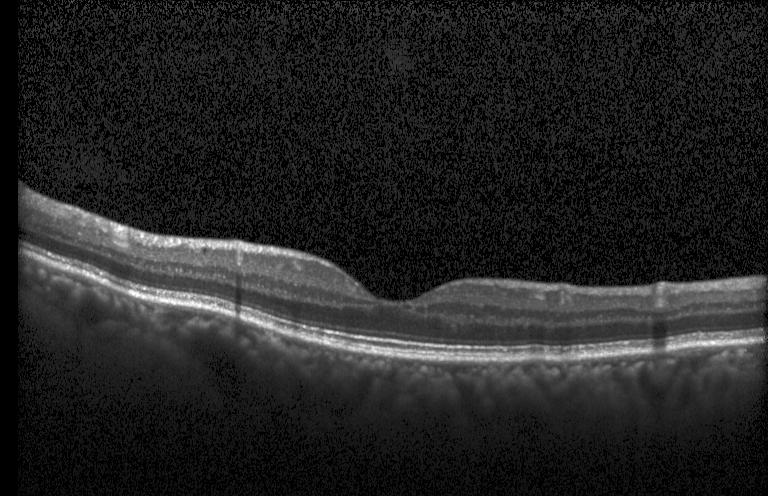
Spectral-domain OCT B-scan: no CNV, no DME, and no drusen.